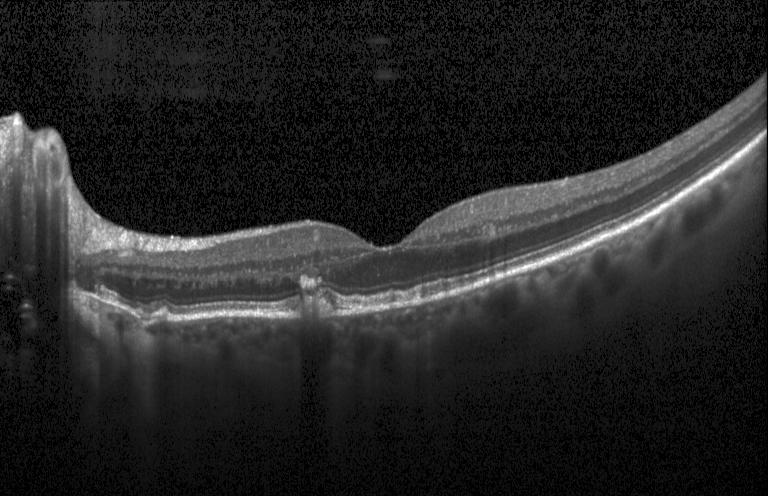

OCT finding: drusen.